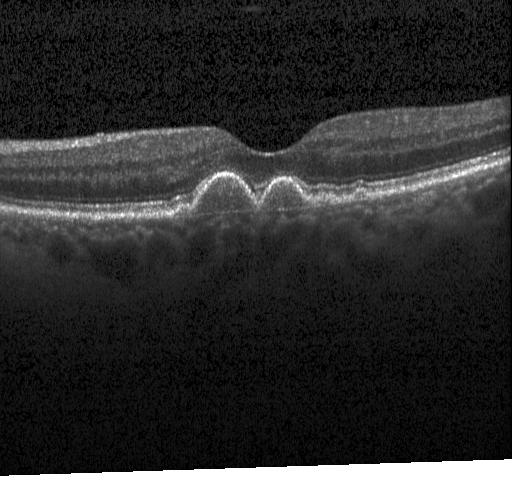
The scan shows sub-RPE drusenoid deposits.